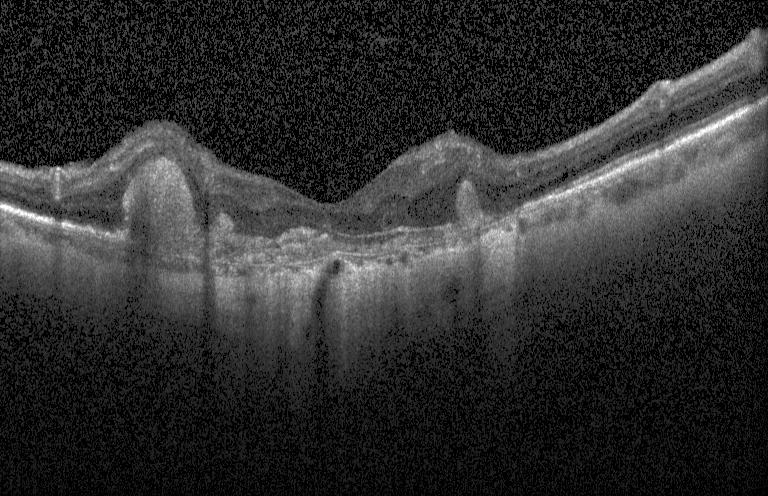 Optical coherence tomography B-scan · spectral-domain optical coherence tomography · Heidelberg Spectralis.
CNV.